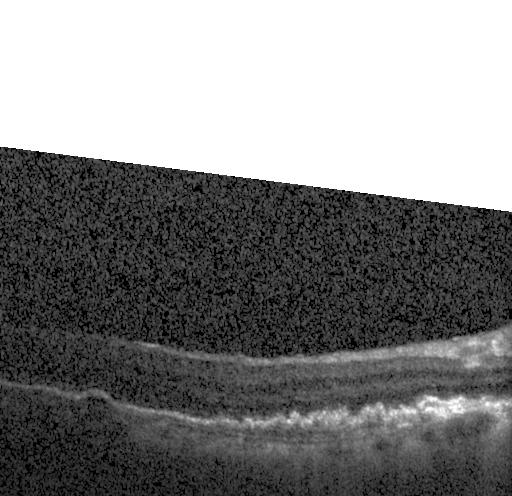 Macular scan · OCT line scan · spectral-domain optical coherence tomography.
This B-scan demonstrates a choroidal neovascular membrane.